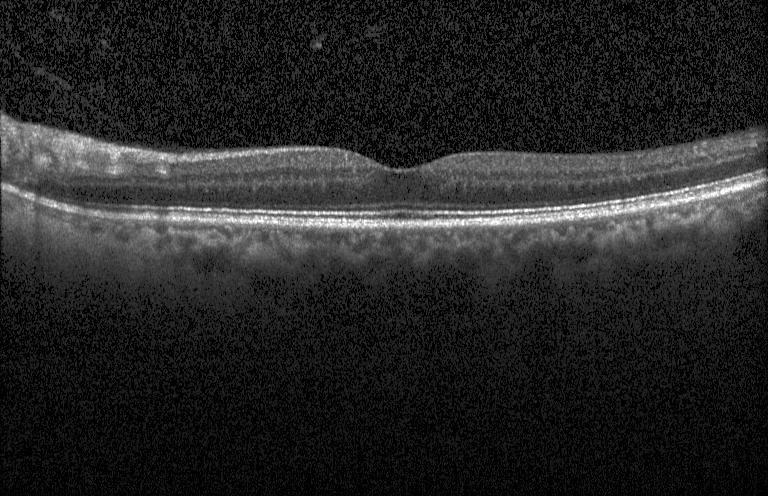 Impression: no CNV, DME, or drusen.